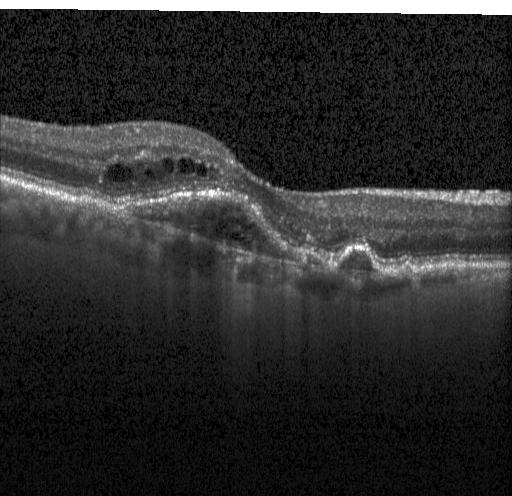
Impression: choroidal neovascularization.